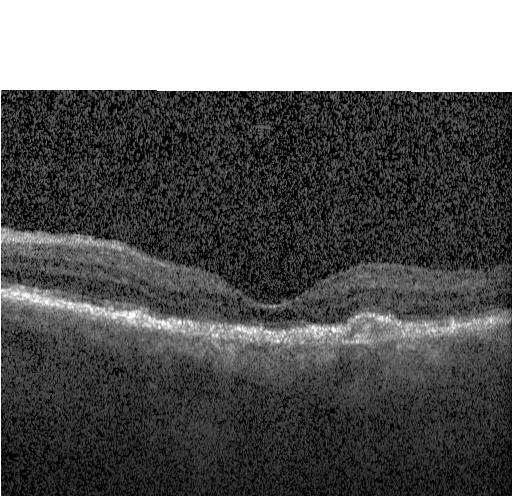

Spectral-domain optical coherence tomography; retinal OCT B-scan.
Impression: choroidal neovascularization.